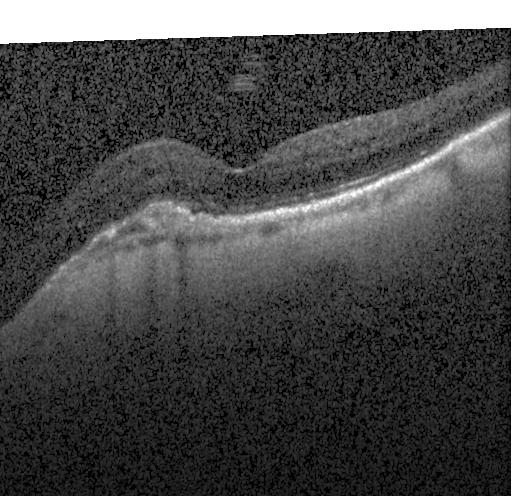
SD-OCT. Instrument: Heidelberg Spectralis. OCT line scan — Finding: choroidal neovascularization.